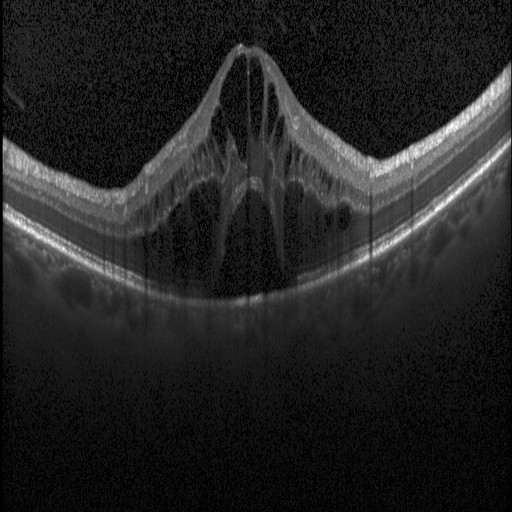

Heidelberg Spectralis OCT system; retinal OCT cross-section; SD-OCT — The scan shows diabetic macular edema (DME).